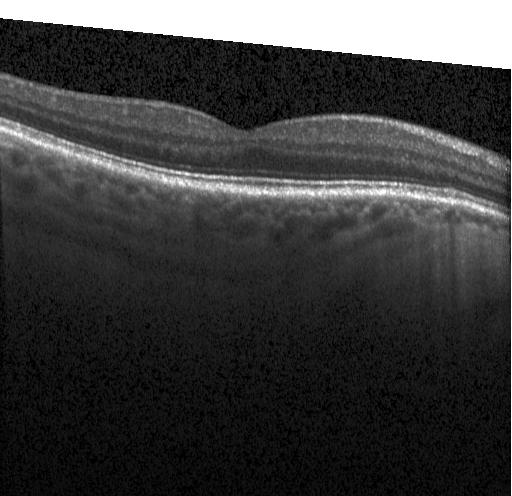 Optical coherence tomography B-scan. SD-OCT. Instrument: Heidelberg Spectralis.
The scan shows neither choroidal neovascularization, diabetic macular edema, nor drusen.